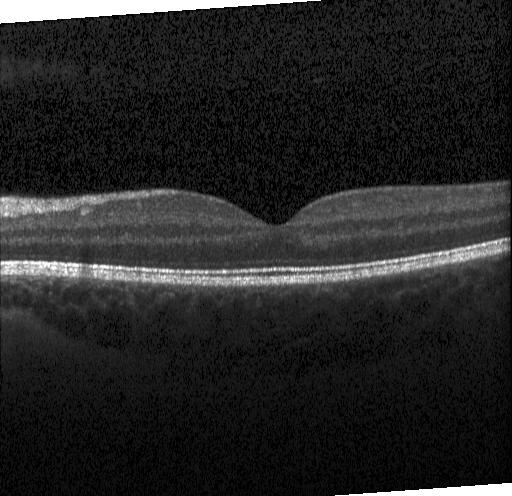

OCT line scan.
Diagnosis: neither choroidal neovascularization, diabetic macular edema, nor drusen.